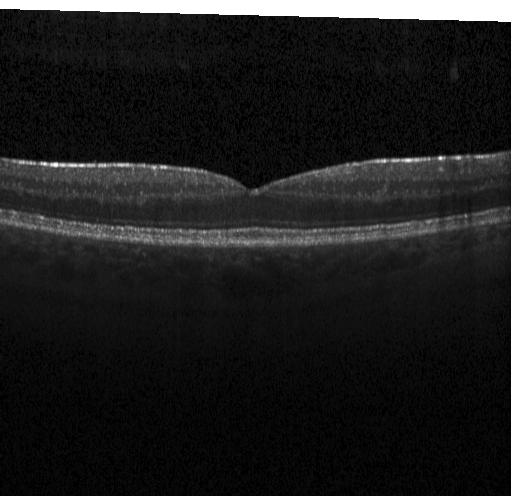 OCT line scan — This B-scan demonstrates no choroidal neovascularization, diabetic macular edema, or drusen.